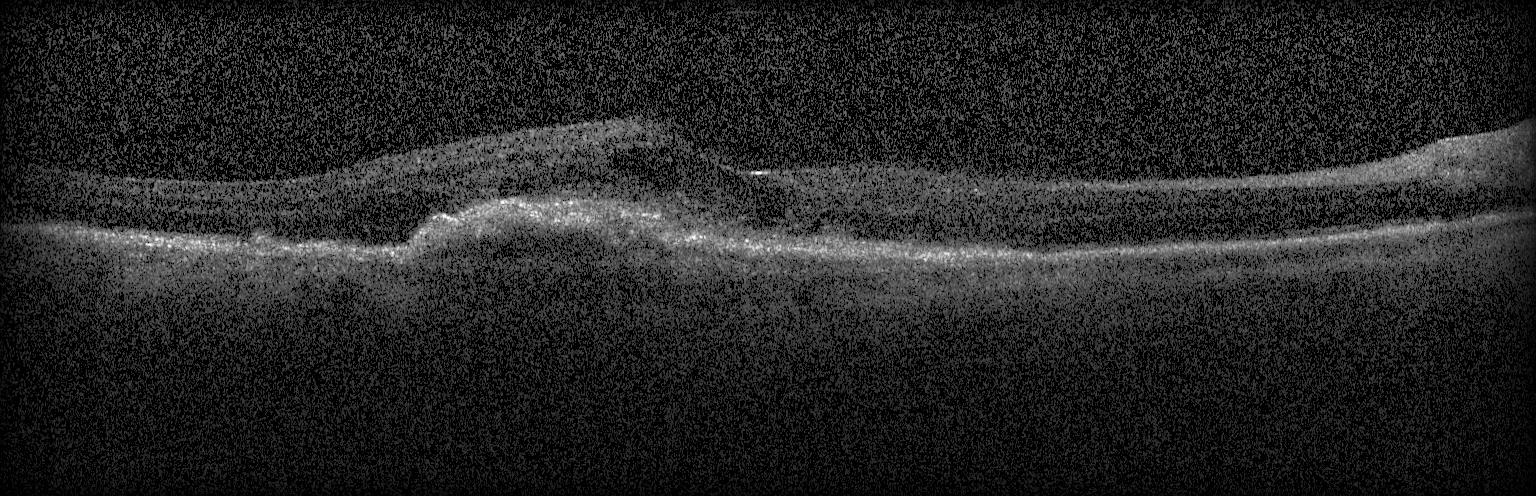 Spectral-domain OCT · Heidelberg Spectralis · OCT line scan · horizontal scan through the fovea. Impression: a choroidal neovascular membrane.